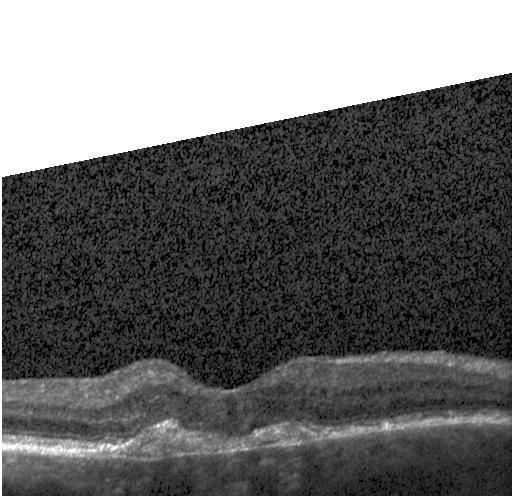

Through the macula. Optical coherence tomography B-scan
Diagnosis: CNV.